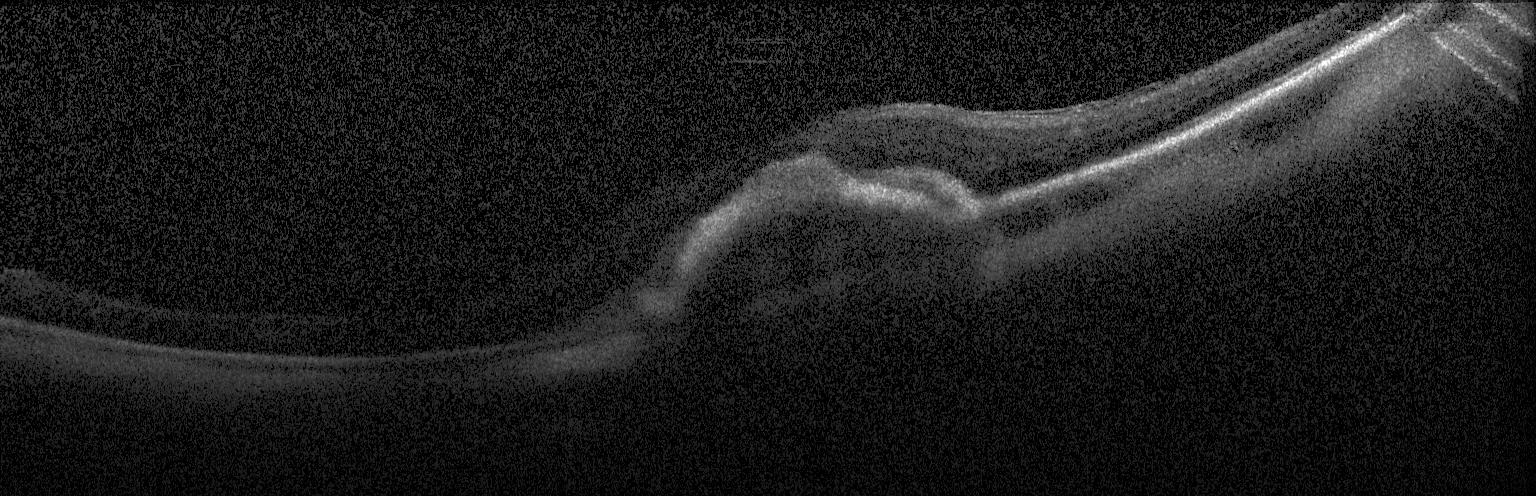 Impression: choroidal neovascularization.